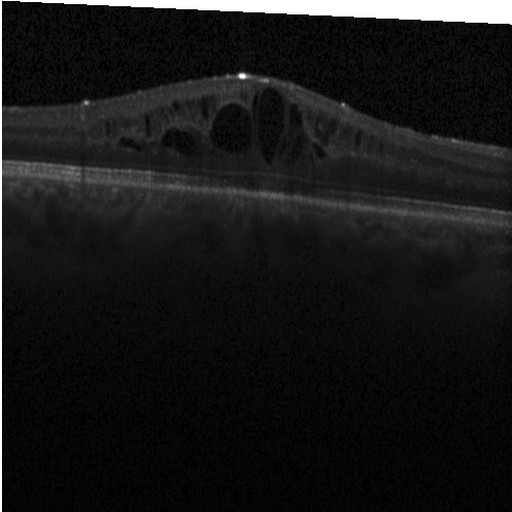 OCT finding: diabetic macular edema (DME).